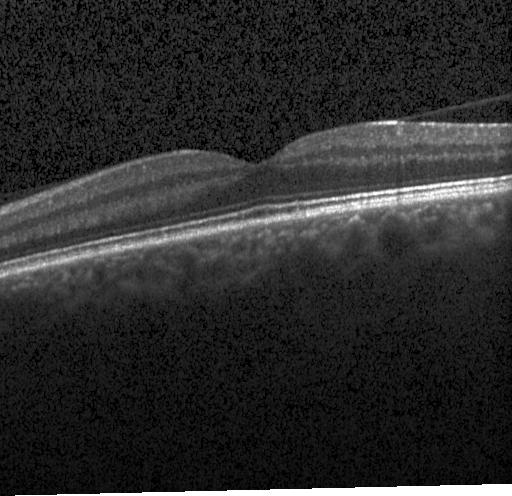
OCT B-scan; Heidelberg Spectralis — Macular OCT: no CNV, no DME, and no drusen.